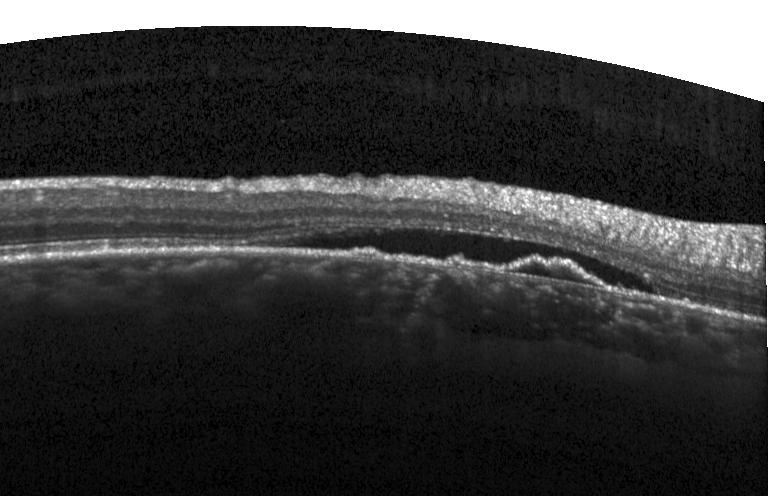 Finding: a choroidal neovascular membrane.